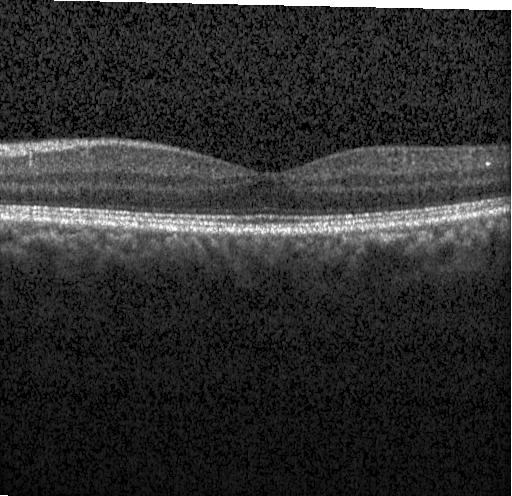 No choroidal neovascularization, diabetic macular edema, or drusen.